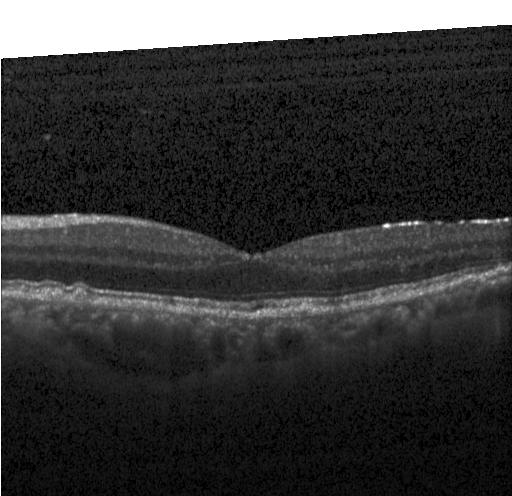 Horizontal scan through the fovea, OCT B-scan, Heidelberg Spectralis OCT system — The scan shows multiple drusen.